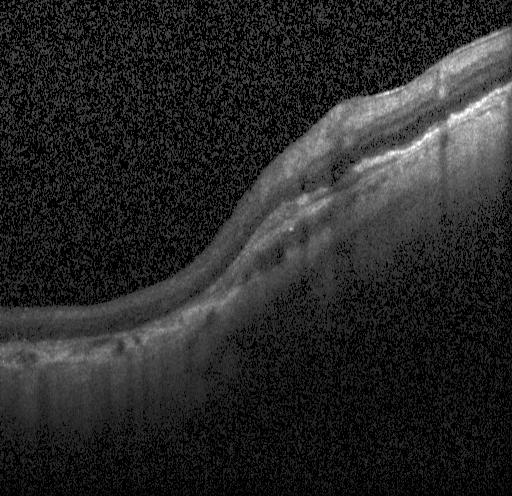 Horizontal scan through the fovea · spectral-domain OCT · retinal OCT B-scan — Finding: CNV.